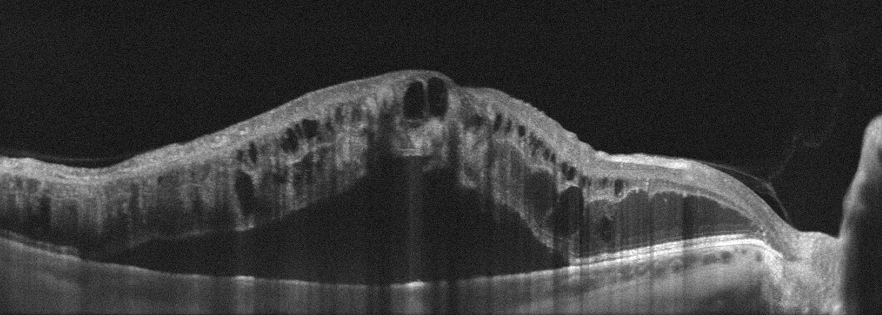

Finding: retinal vein occlusion.